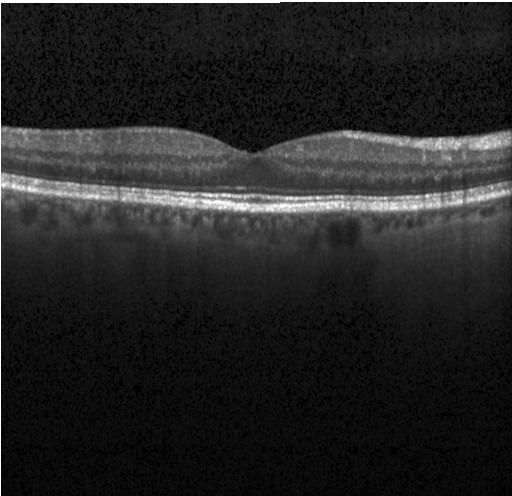
Retinal OCT cross-section. Diagnosis: no choroidal neovascularization, no diabetic macular edema, and no drusen.